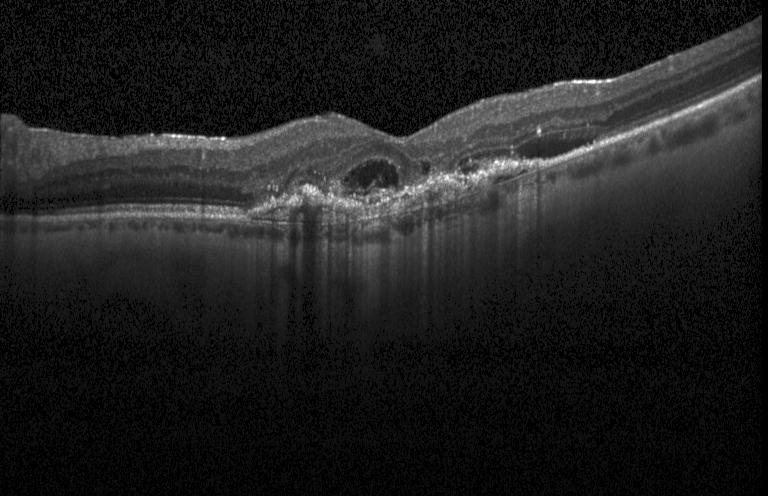

OCT B-scan; through the macula; spectral-domain optical coherence tomography. Diagnosis: choroidal neovascularization.